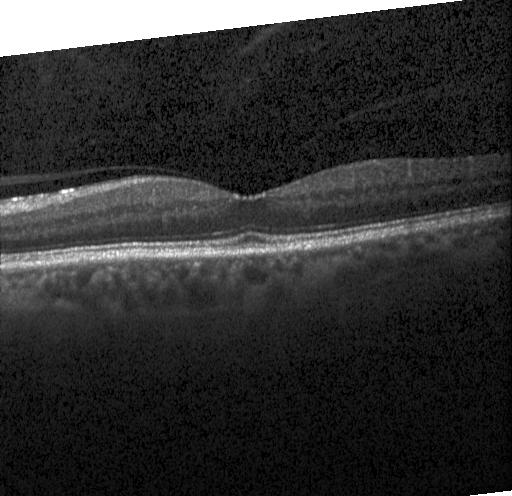 Optical coherence tomography scan.
This B-scan demonstrates no choroidal neovascularization, diabetic macular edema, or drusen.